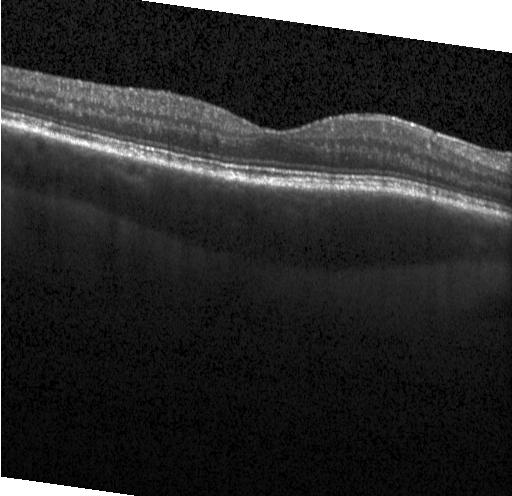
Finding: neither choroidal neovascularization, diabetic macular edema, nor drusen.